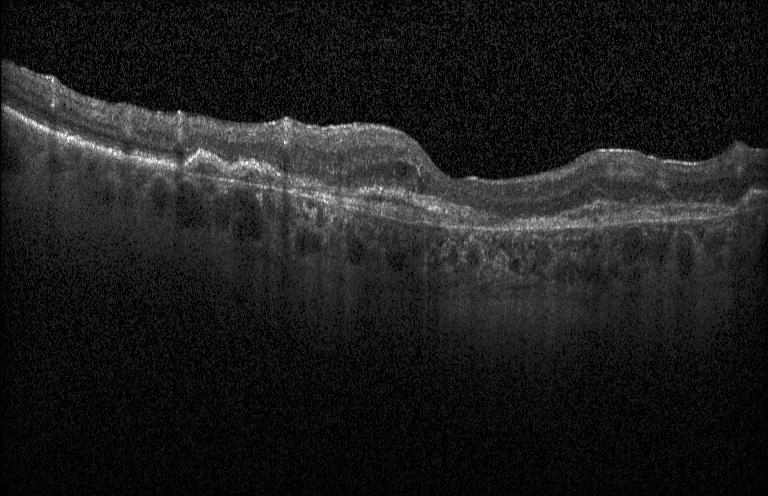 Macular OCT demonstrating choroidal neovascularization (CNV).